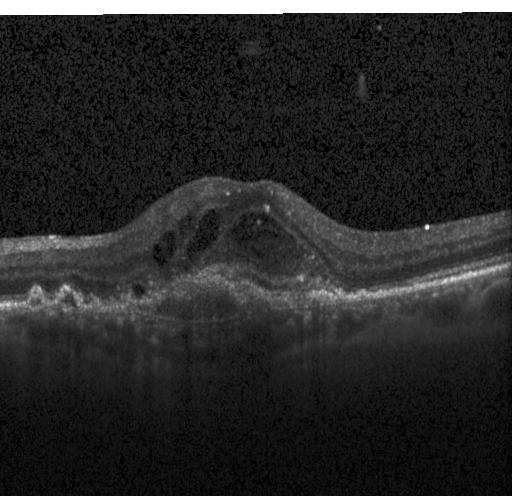 Spectral-domain OCT B-scan: CNV.